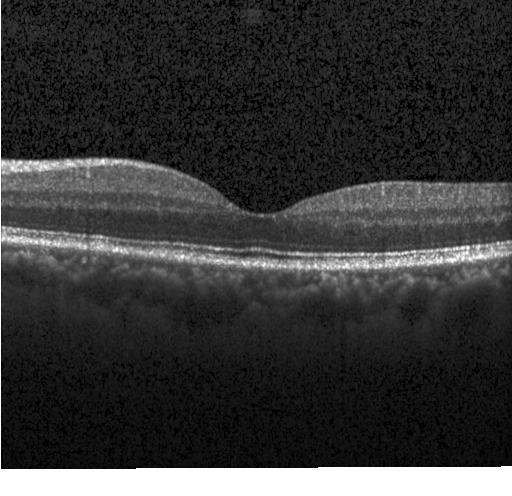 Macular OCT demonstrating no evidence of choroidal neovascularization, diabetic macular edema, or drusen.